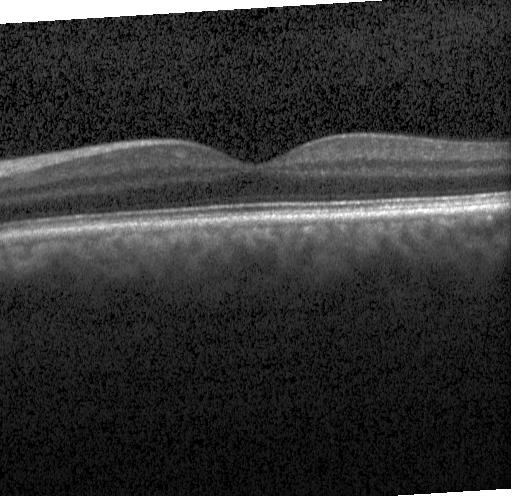

OCT scan showing no choroidal neovascularization, diabetic macular edema, or drusen.